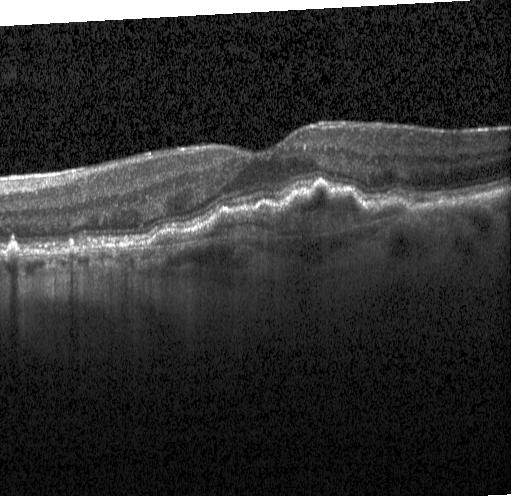
Diagnosis: choroidal neovascularization.